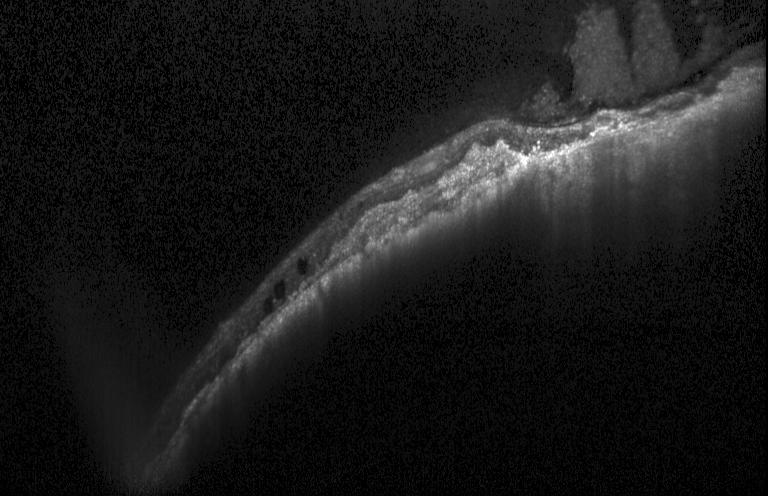
OCT B-scan. Dx: CNV.